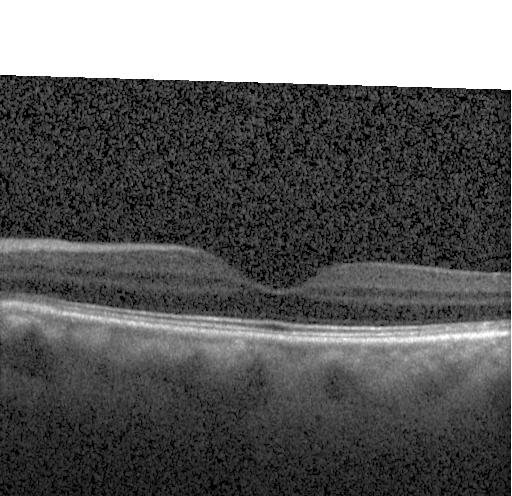

Retinal OCT cross-section showing no evidence of choroidal neovascularization, diabetic macular edema, or drusen.